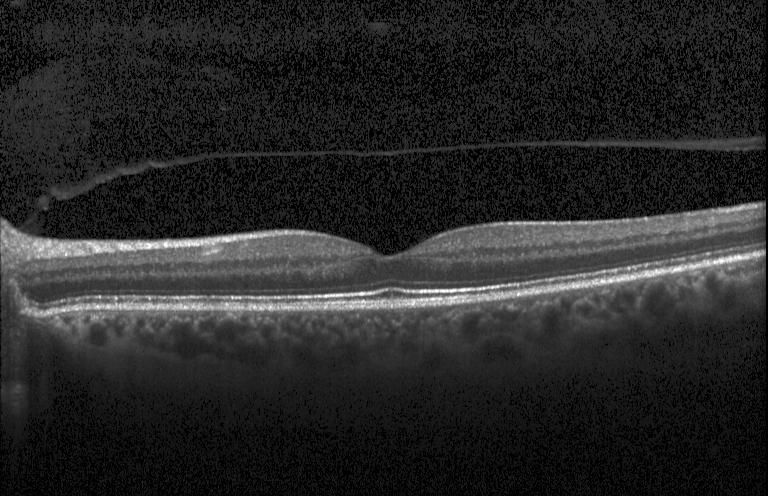 Optical coherence tomography scan · Heidelberg Spectralis · centered on the fovea · SD-OCT. Assessment: no evidence of CNV, DME, or drusen.